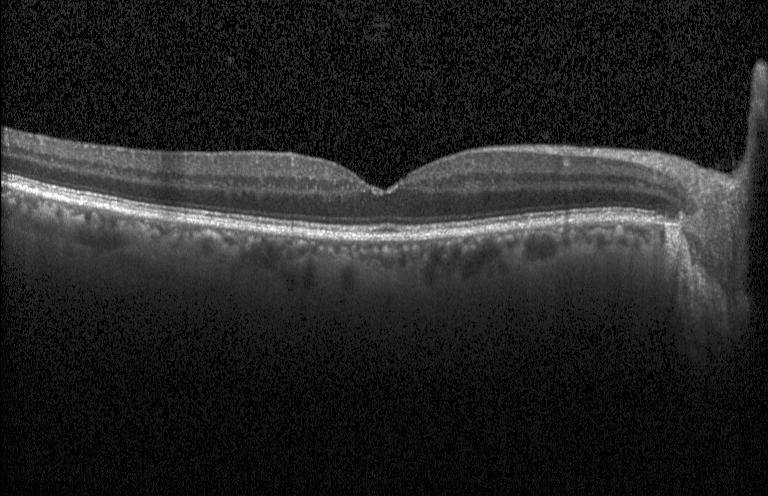 OCT B-scan · spectral-domain optical coherence tomography.
Dx: no evidence of choroidal neovascularization, diabetic macular edema, or drusen.